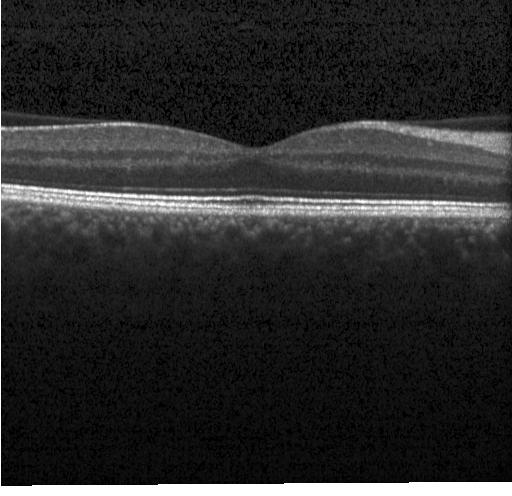

Acquired on a Heidelberg Spectralis, retinal OCT cross-section, spectral-domain optical coherence tomography — Finding: no evidence of CNV, DME, or drusen.